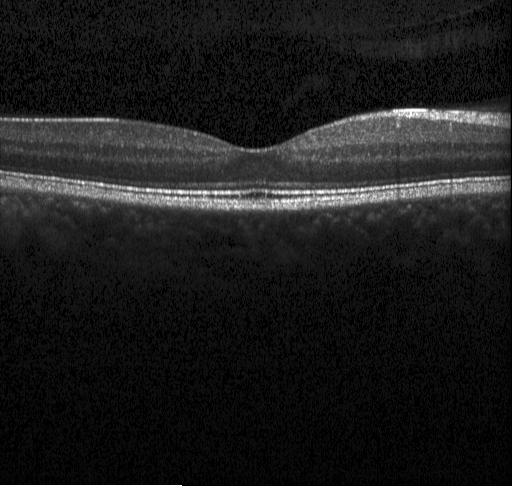

OCT B-scan — Impression: neither choroidal neovascularization, diabetic macular edema, nor drusen.